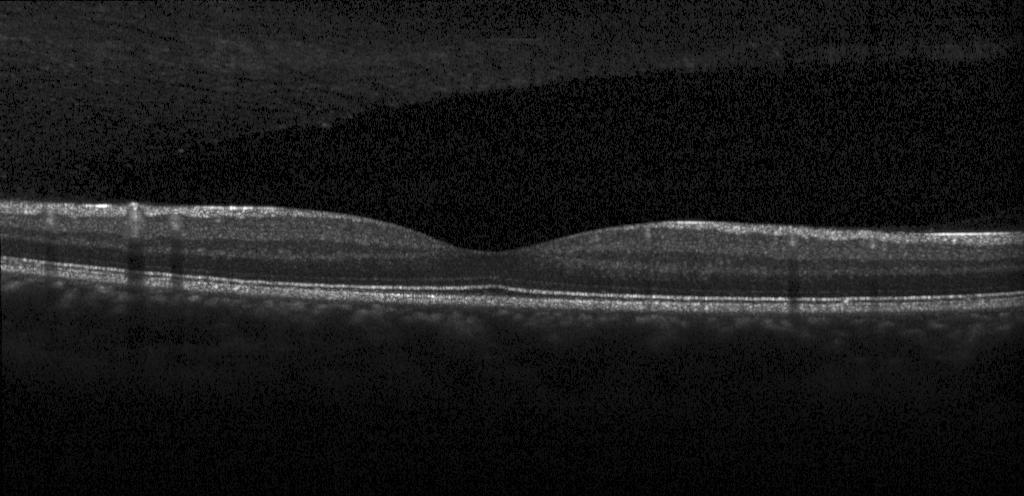
No evidence of CNV, DME, or drusen.